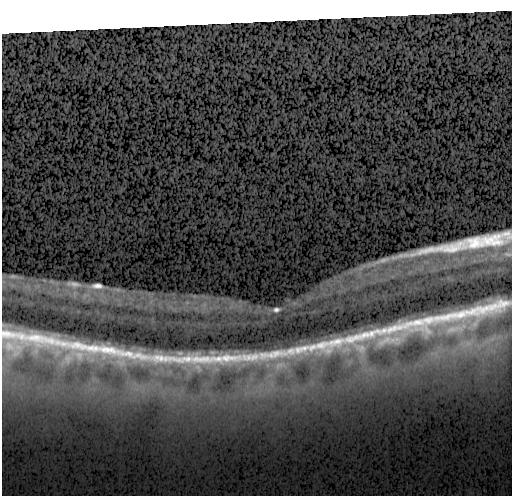 Retinal OCT cross-section. Macular scan. Macular OCT: no evidence of CNV, DME, or drusen.